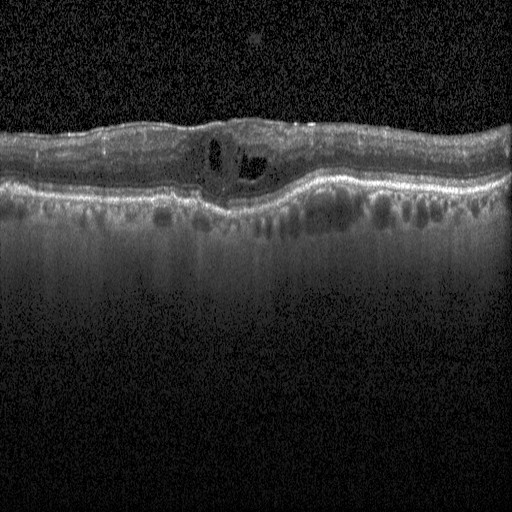 This B-scan demonstrates DME.